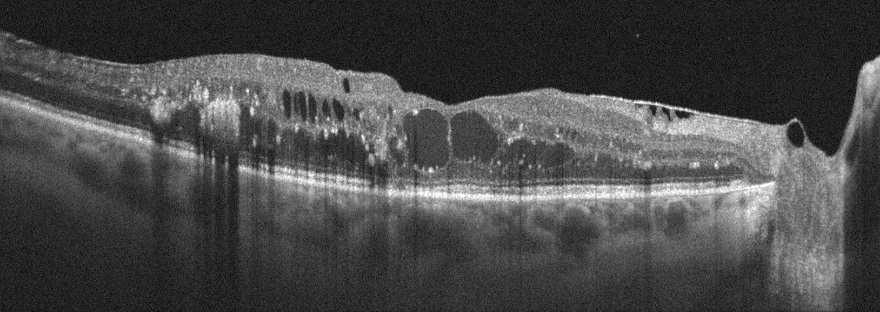

Retinal OCT cross-section showing diabetic macular edema.